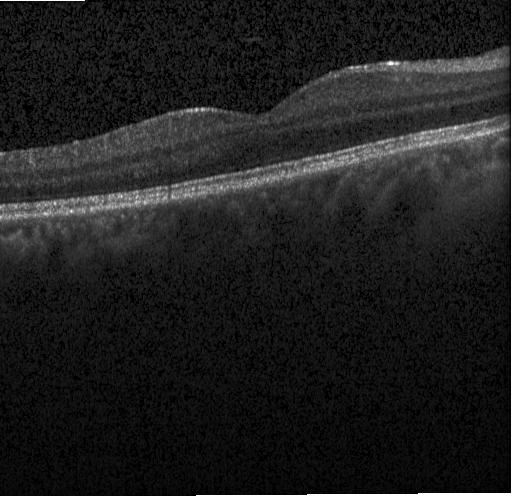 Centered on the fovea · retinal OCT cross-section · instrument: Heidelberg Spectralis · spectral-domain optical coherence tomography
Finding: neither CNV, DME, nor drusen.